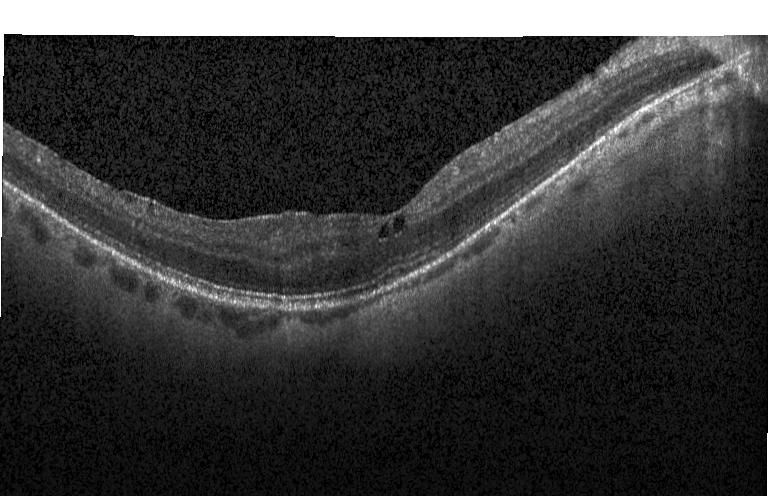
Acquired on a Heidelberg Spectralis · spectral-domain OCT · OCT B-scan — Dx: diabetic macular edema (DME).